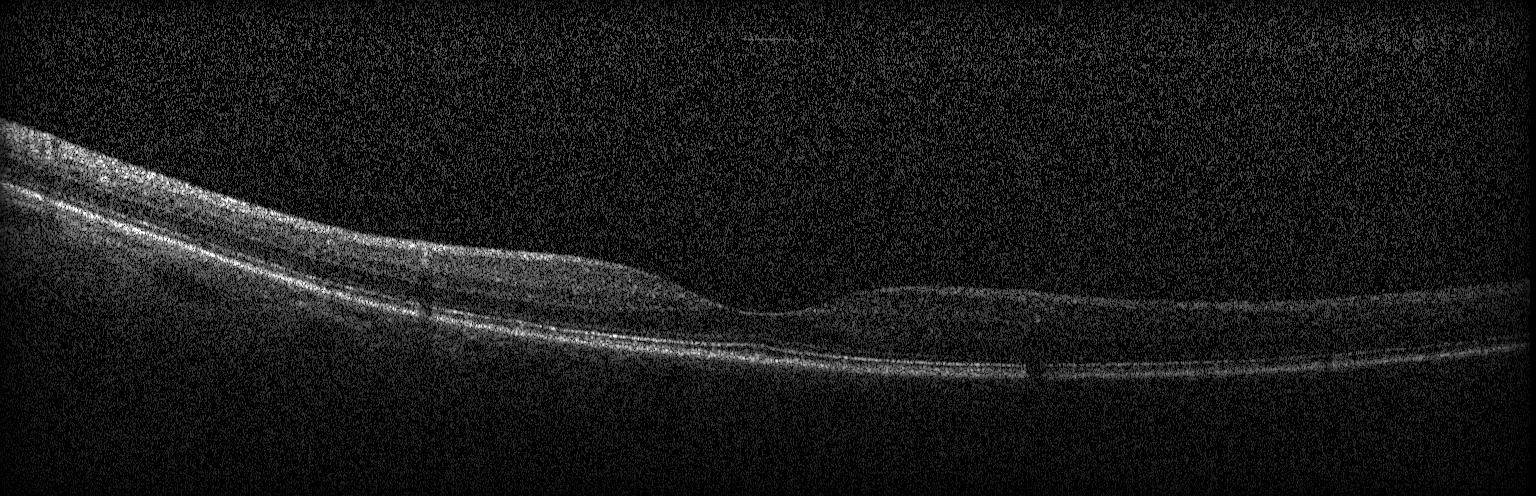
Heidelberg Spectralis. Optical coherence tomography scan — Impression: no CNV, no DME, and no drusen.